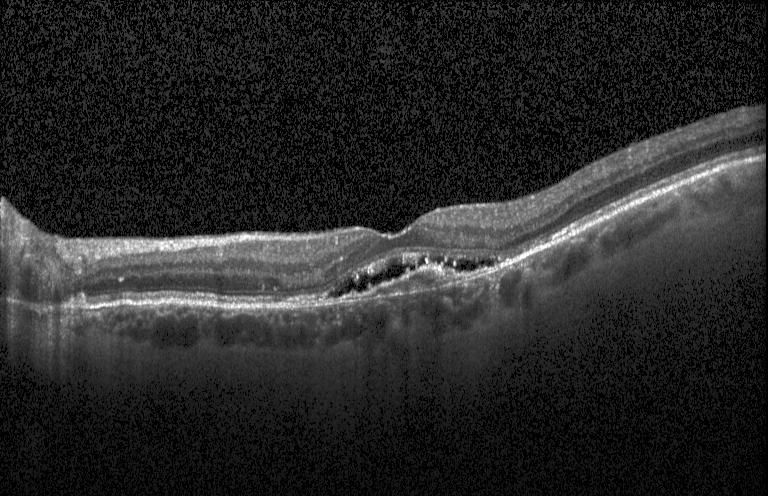 Retinal OCT B-scan. Spectral-domain optical coherence tomography. Impression: CNV.